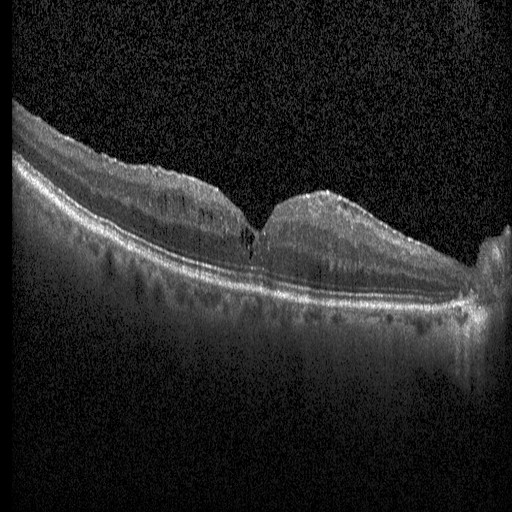
SD-OCT, horizontal scan through the fovea, optical coherence tomography scan — Finding: diabetic macular edema (DME).